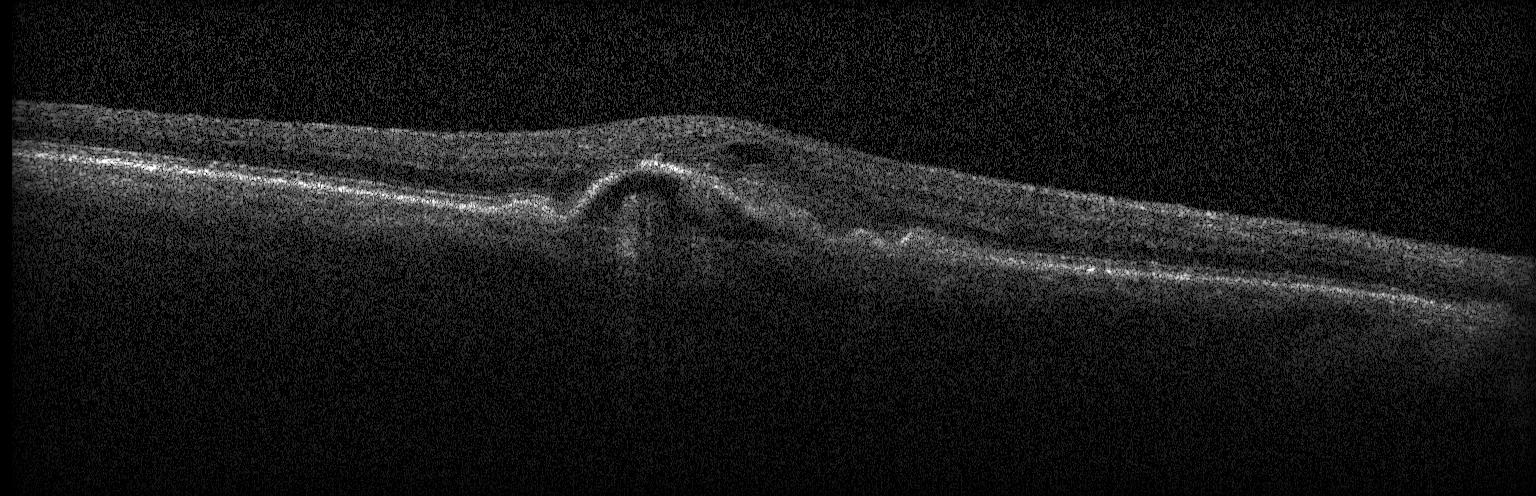 Impression: a choroidal neovascular membrane.